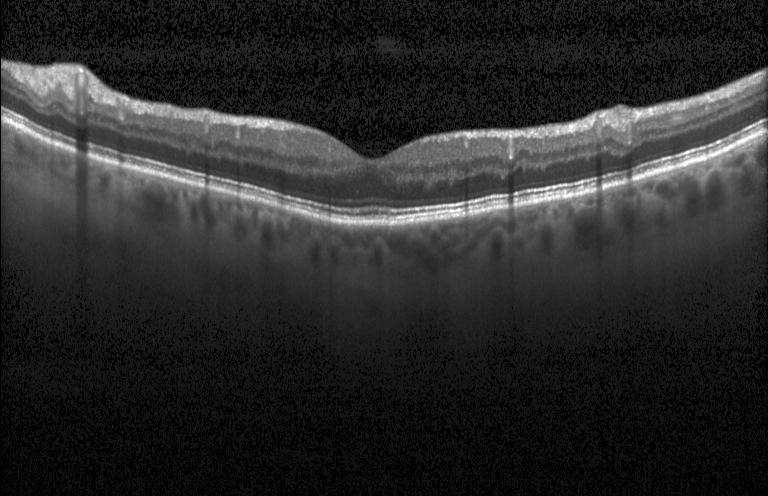
Diagnosis: neither CNV, DME, nor drusen.